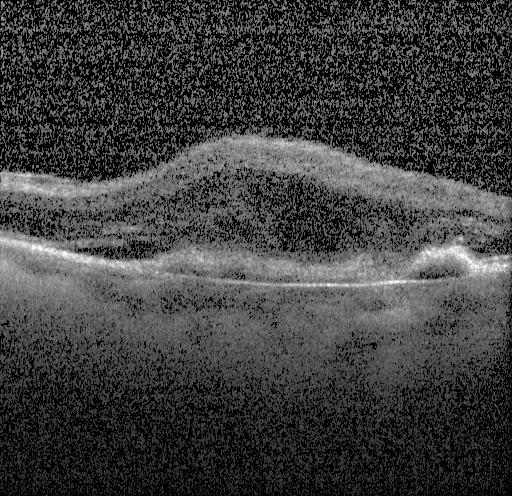

Retinal OCT cross-section showing choroidal neovascularization (CNV).